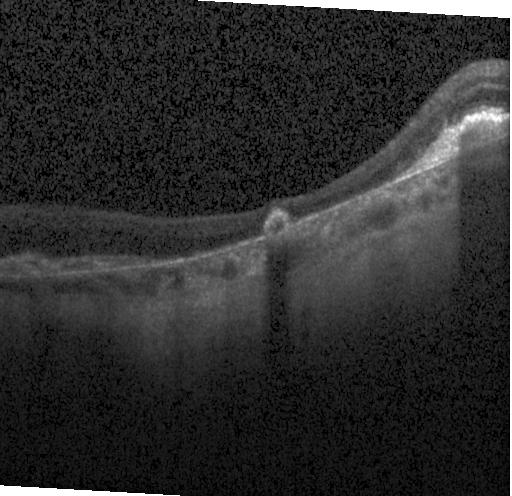
Finding: choroidal neovascularization (CNV).